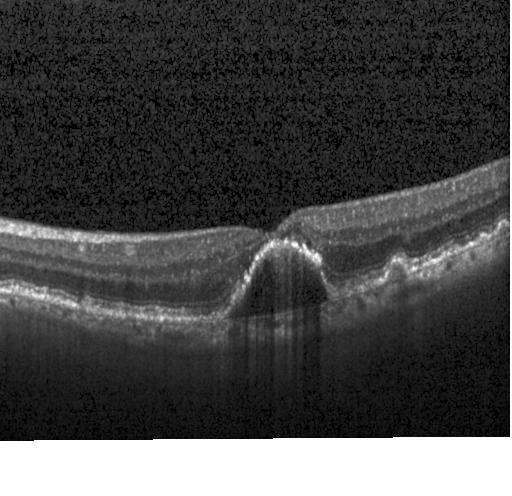 Centered on the fovea. Retinal OCT B-scan. Spectral-domain optical coherence tomography
This B-scan demonstrates a choroidal neovascular membrane.